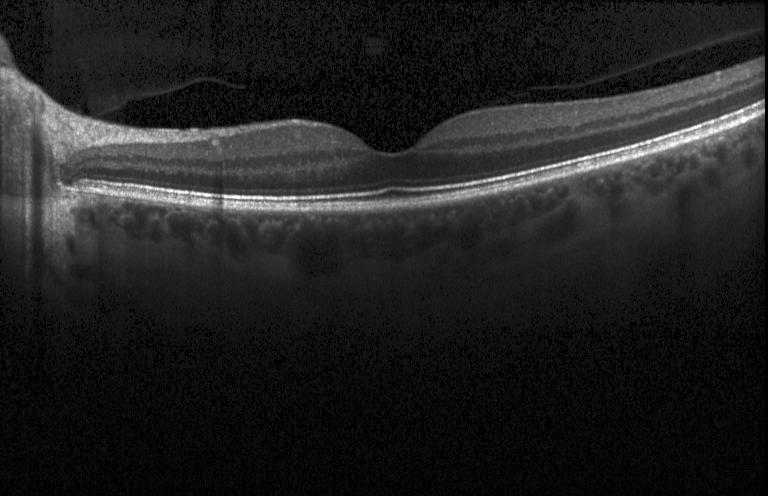
OCT finding: no CNV, DME, or drusen.